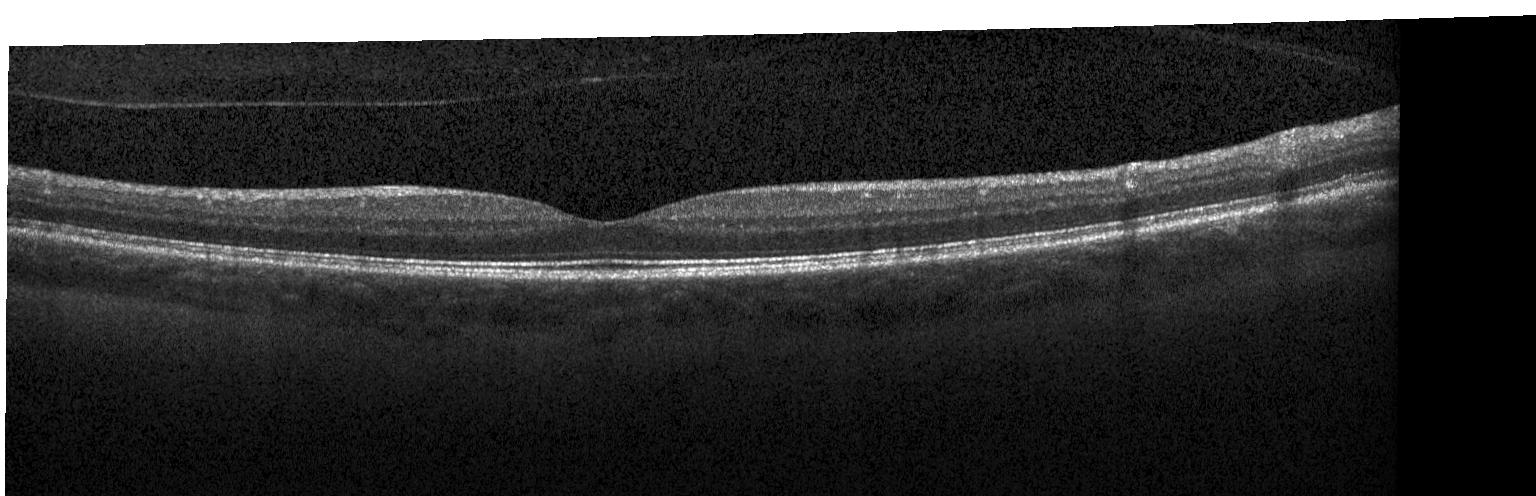 Spectral-domain OCT; centered on the fovea; retinal OCT B-scan. Diagnosis: neither CNV, DME, nor drusen.